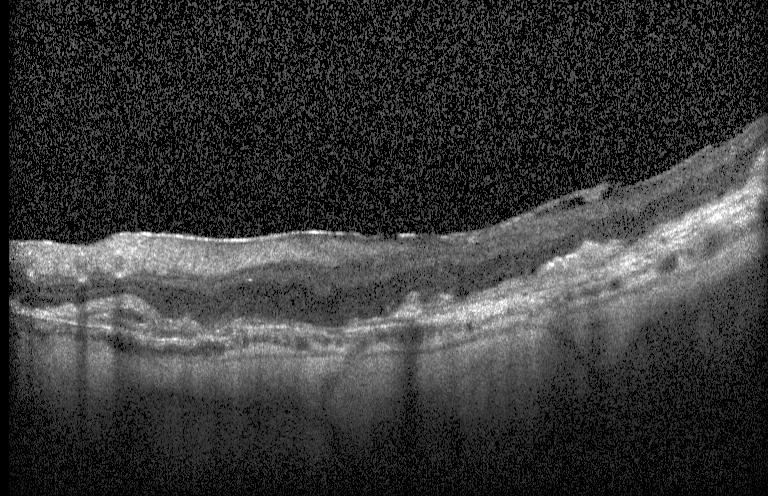
Optical coherence tomography scan — Impression: CNV.